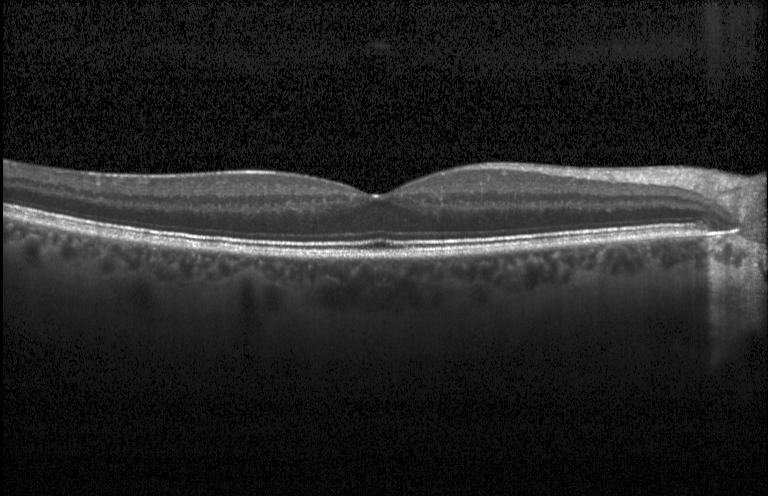
Spectral-domain OCT. Optical coherence tomography B-scan.
Macular OCT: no choroidal neovascularization, diabetic macular edema, or drusen.